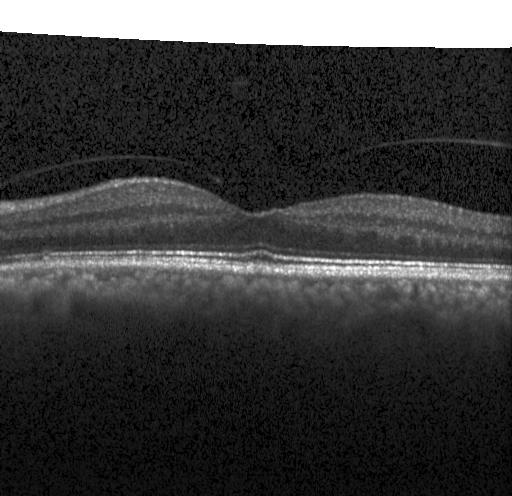 Spectral-domain OCT, centered on the fovea, optical coherence tomography B-scan — Impression: neither CNV, DME, nor drusen.